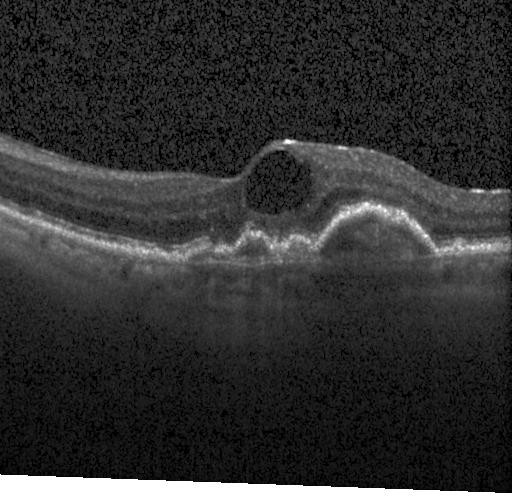

Fovea-centered, Heidelberg Spectralis OCT system, optical coherence tomography scan — Impression: CNV.